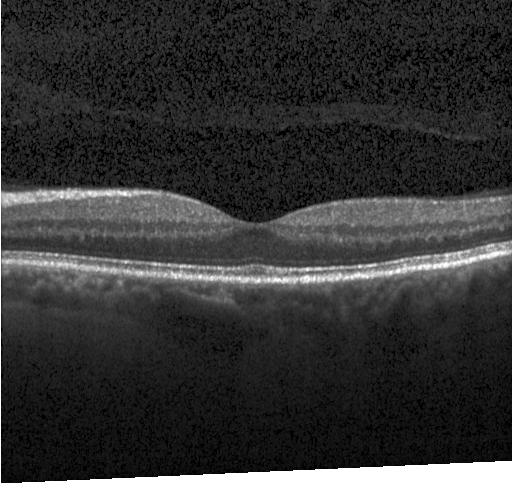

Fovea-centered · SD-OCT · optical coherence tomography scan
Finding: neither choroidal neovascularization, diabetic macular edema, nor drusen.